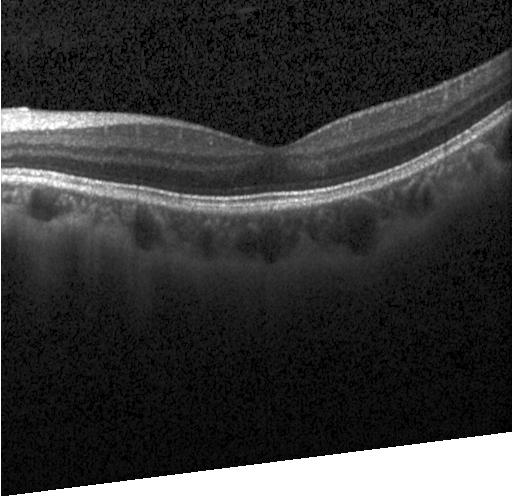

Optical coherence tomography scan; spectral-domain OCT; acquired on a Heidelberg Spectralis; fovea-centered — Assessment: no choroidal neovascularization, diabetic macular edema, or drusen.